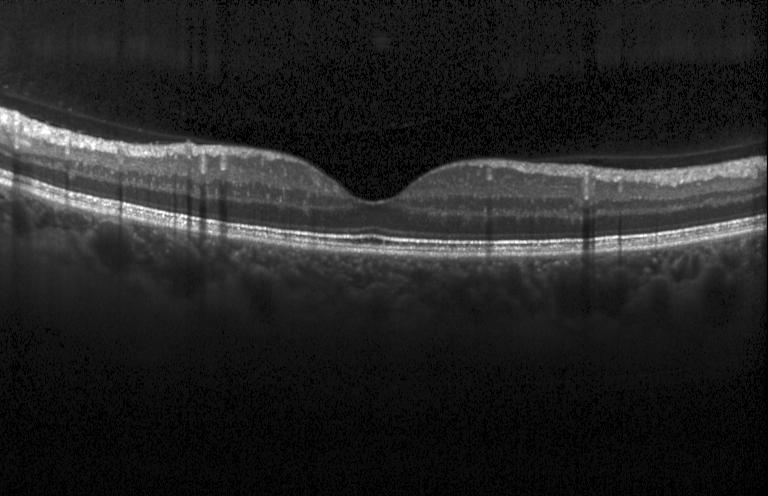

Diagnosis: no CNV, DME, or drusen.